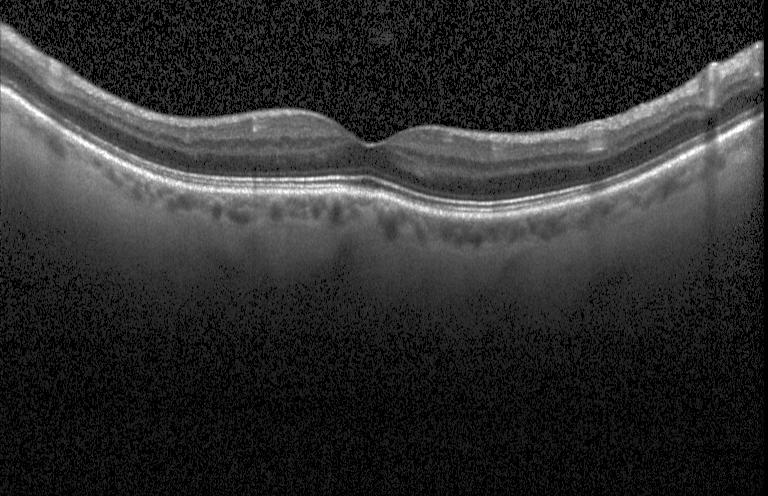
Spectral-domain optical coherence tomography; Heidelberg Spectralis; OCT B-scan — Macular OCT: no CNV, DME, or drusen.